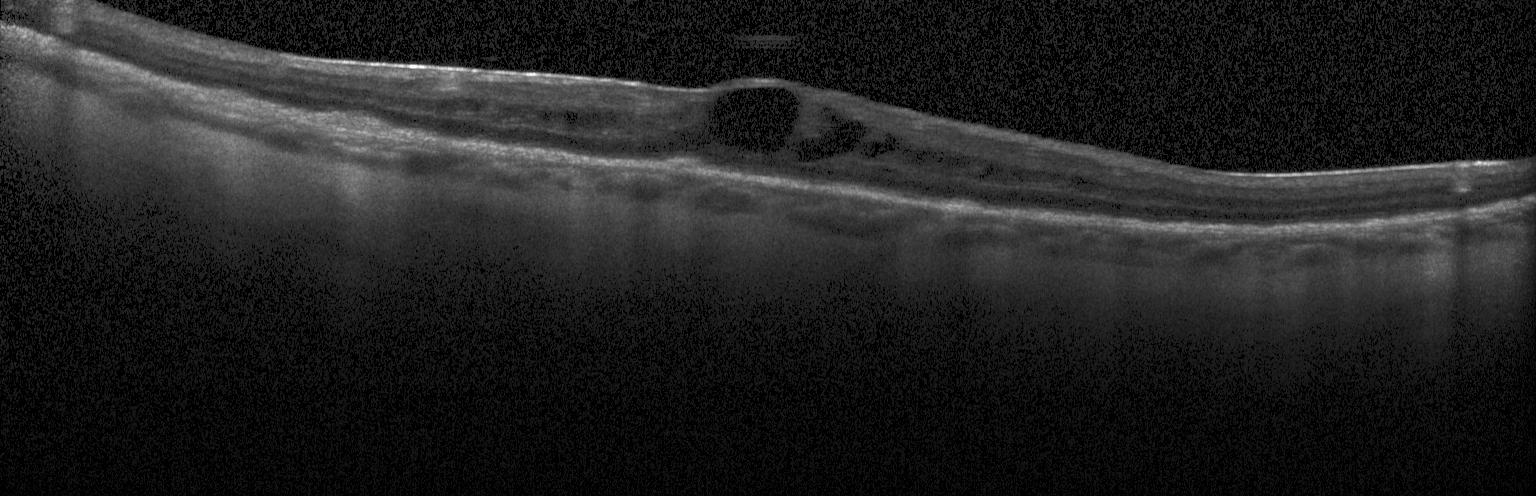 OCT B-scan; spectral-domain OCT; through the macula; Heidelberg Spectralis.
Impression: a choroidal neovascular membrane.